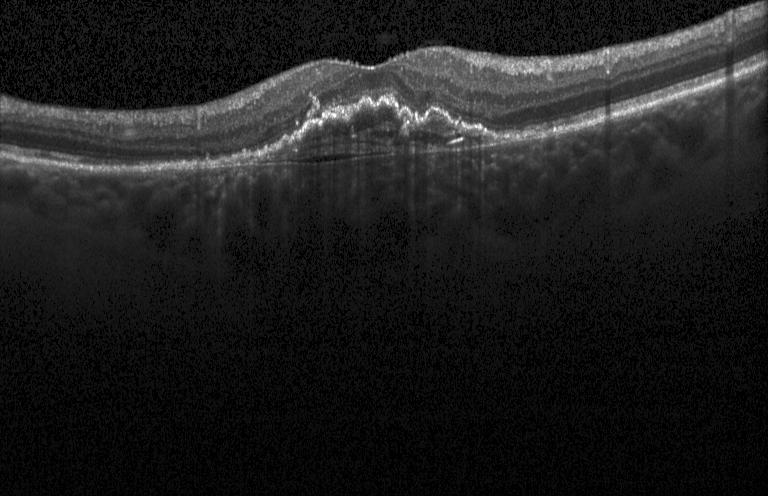 Retinal OCT cross-section. The scan shows a choroidal neovascular membrane.